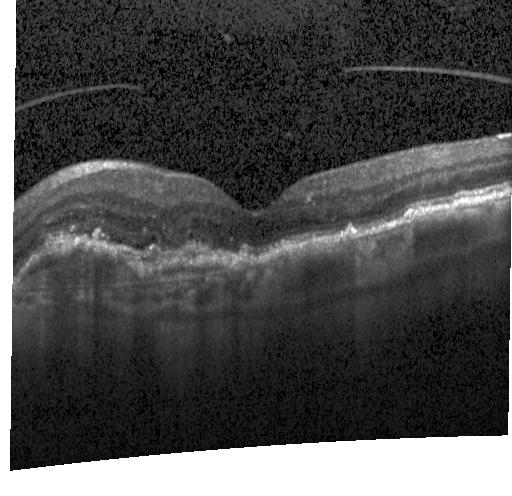 Macular scan, spectral-domain optical coherence tomography, acquired on a Heidelberg Spectralis, optical coherence tomography scan. Impression: choroidal neovascularization.